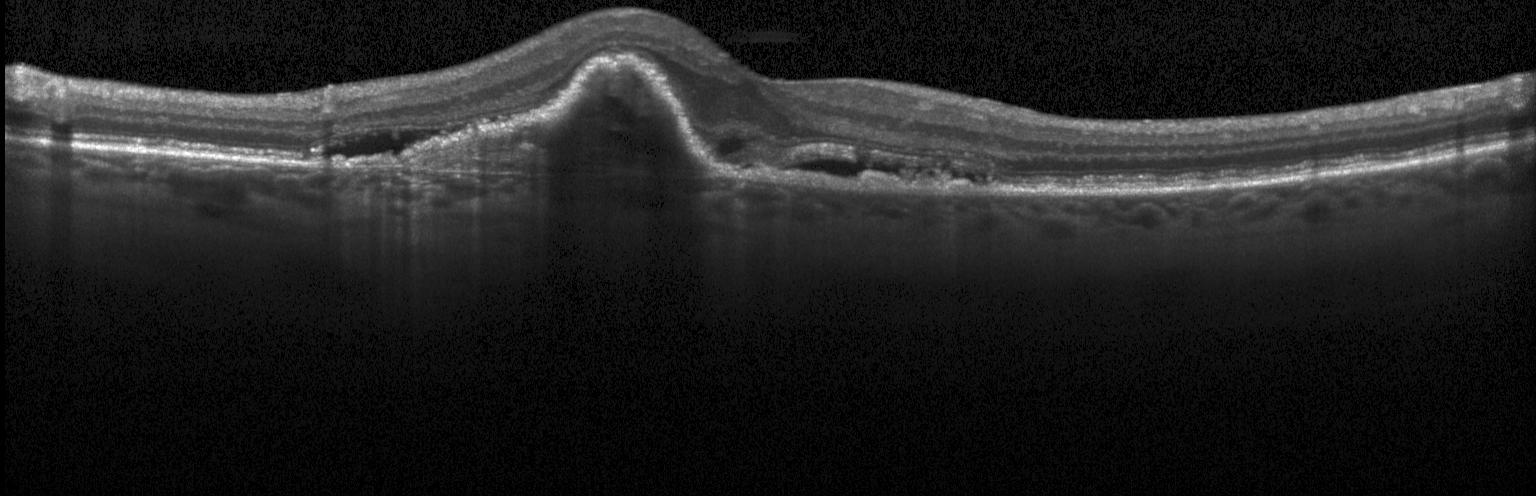
OCT B-scan. Heidelberg Spectralis
Finding: a choroidal neovascular membrane.